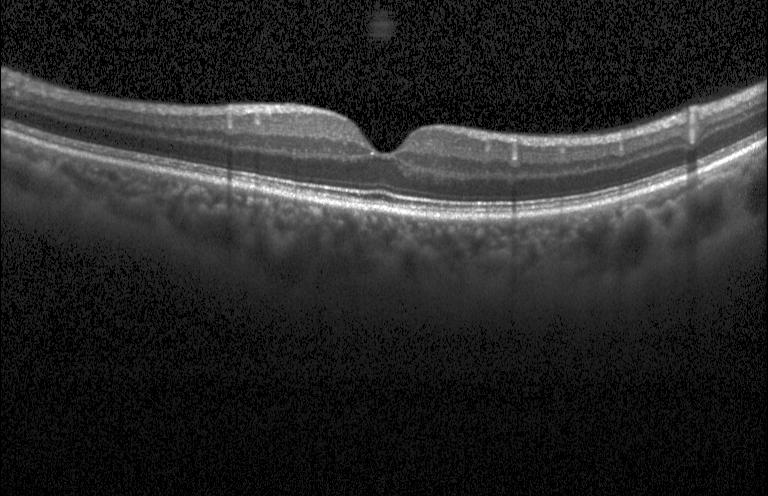
Retinal OCT cross-section showing no CNV, DME, or drusen.